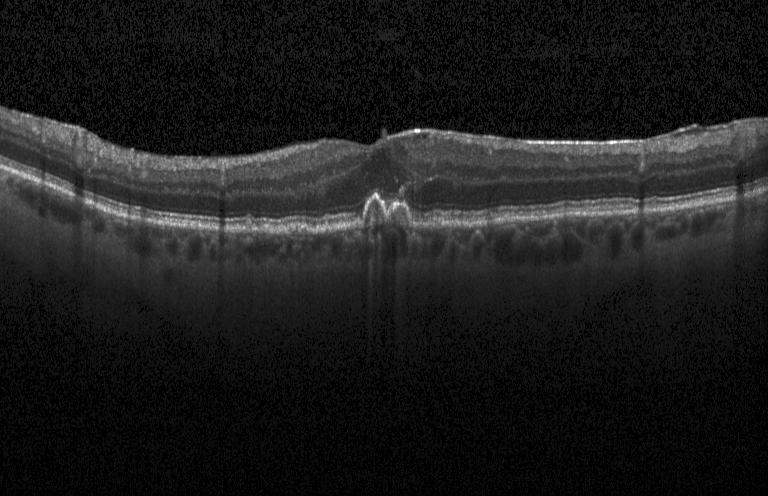
Optical coherence tomography B-scan, spectral-domain OCT, macular scan.
Impression: multiple drusen.